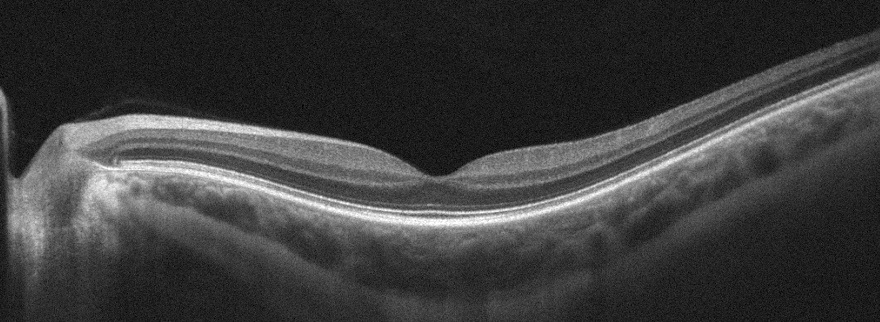
OCT B-scan showing no AMD, DME, ERM, RAO, RVO, or VID.